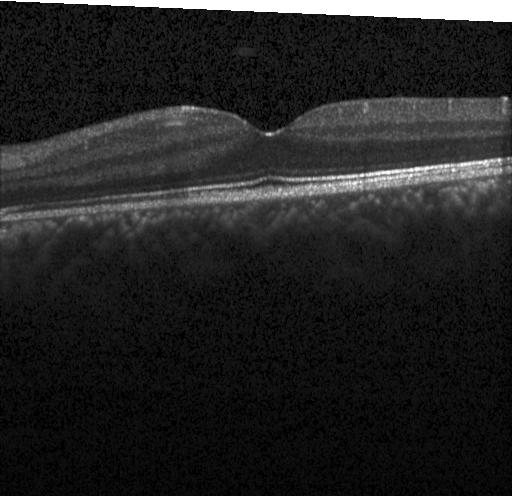

Instrument: Heidelberg Spectralis; horizontal scan through the fovea; retinal OCT B-scan; spectral-domain optical coherence tomography. This B-scan demonstrates neither choroidal neovascularization, diabetic macular edema, nor drusen.